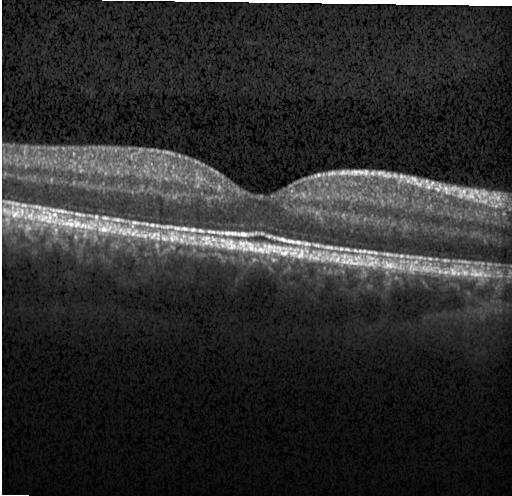
Instrument: Heidelberg Spectralis; OCT line scan — Diagnosis: neither CNV, DME, nor drusen.